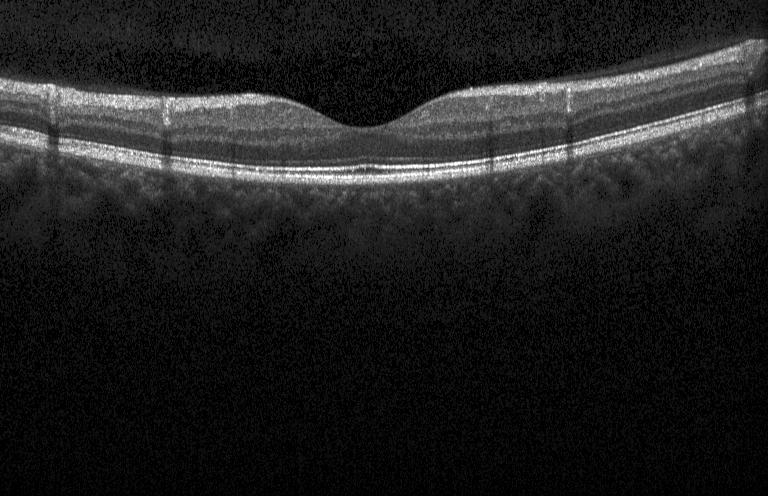

OCT scan showing neither choroidal neovascularization, diabetic macular edema, nor drusen.